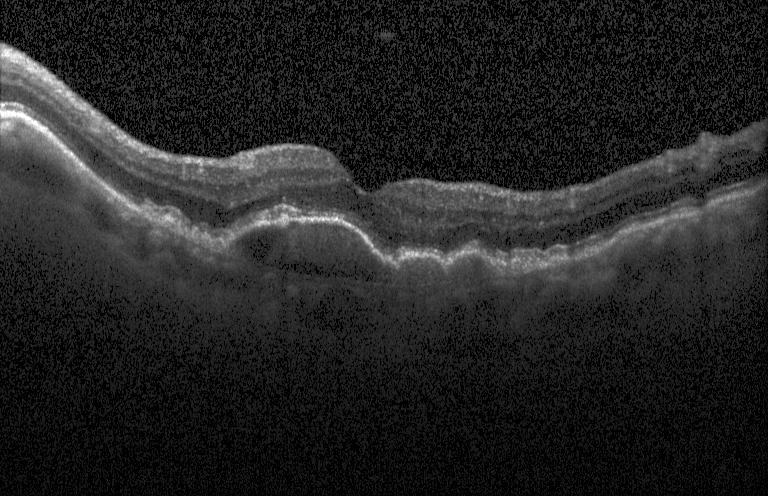
Optical coherence tomography B-scan, instrument: Heidelberg Spectralis
Finding: sub-RPE drusenoid deposits.